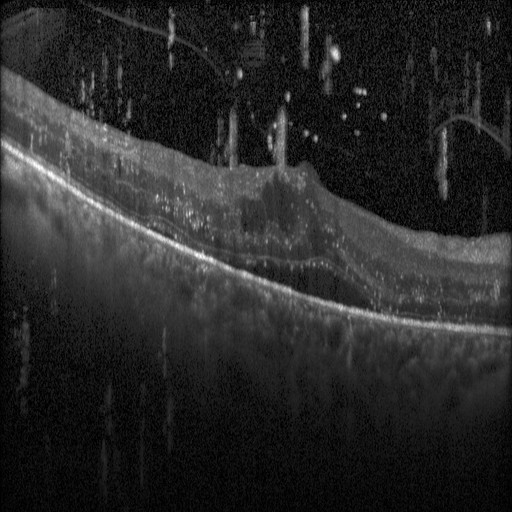 Macular OCT demonstrating diabetic macular edema (DME).